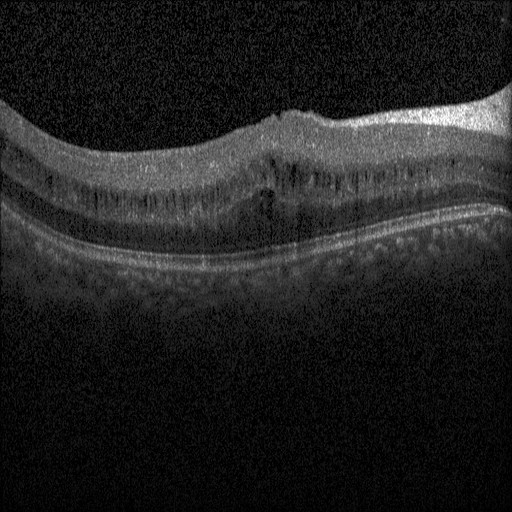 Fovea-centered, optical coherence tomography scan, SD-OCT. Impression: DME.